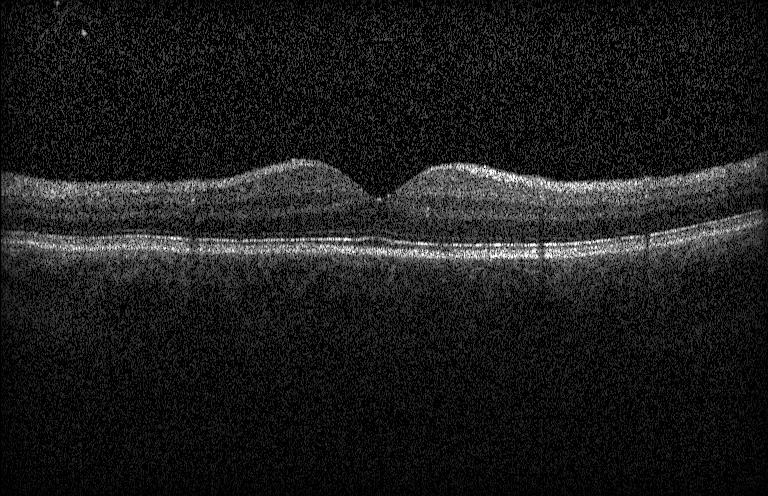 Heidelberg Spectralis, OCT line scan, centered on the fovea, SD-OCT
OCT finding: no CNV, no DME, and no drusen.